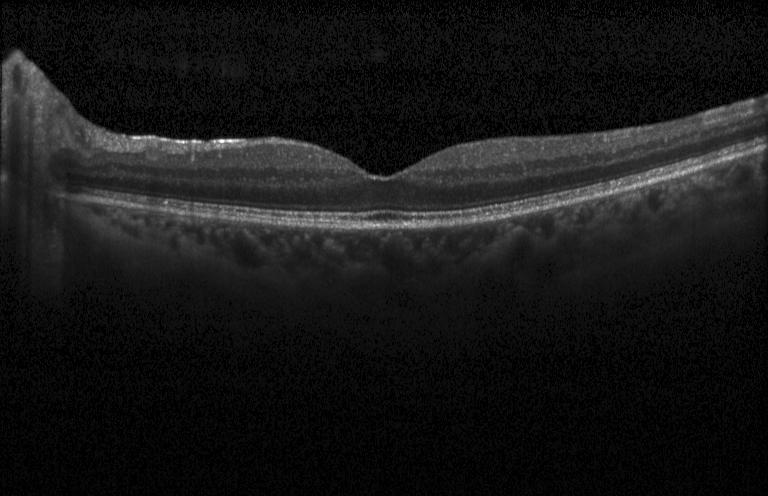
This B-scan demonstrates no CNV, DME, or drusen.